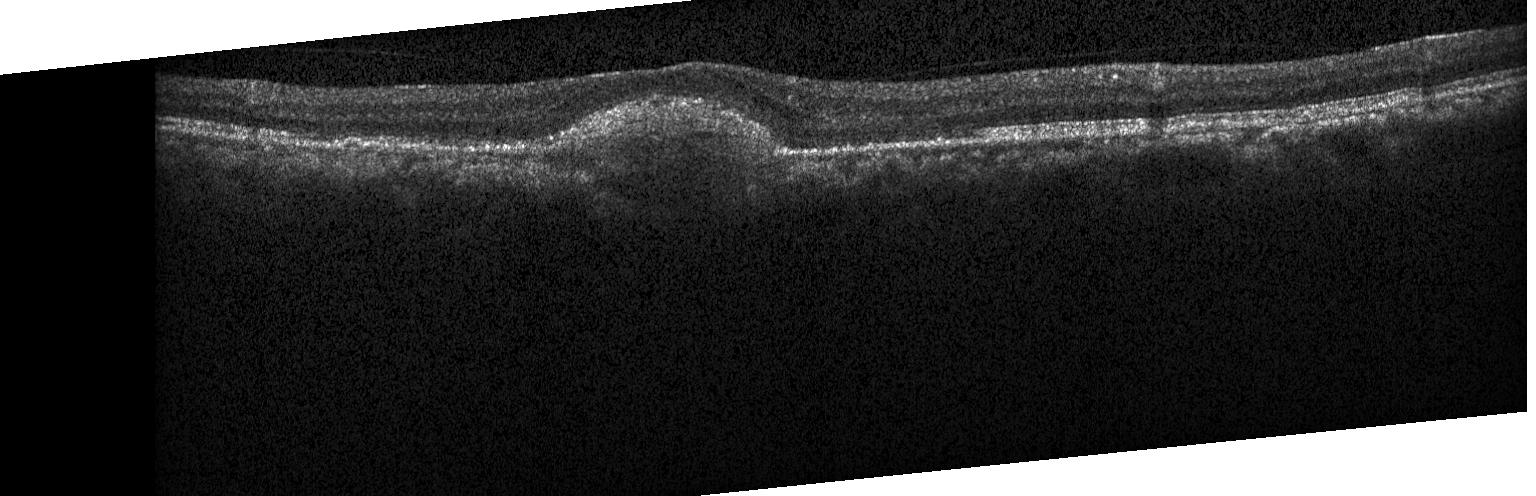

This B-scan demonstrates choroidal neovascularization.